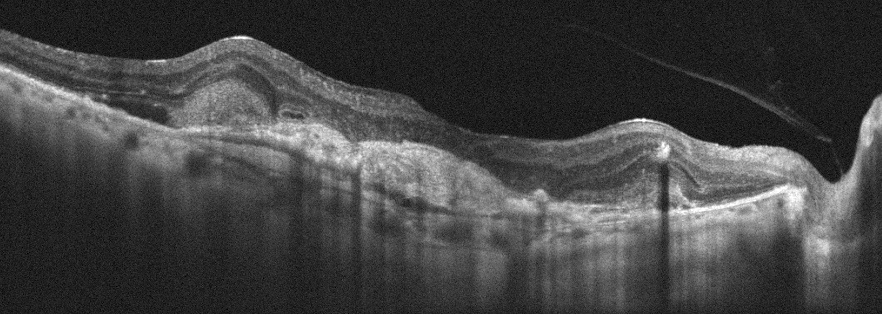

Age-related macular degeneration (AMD).